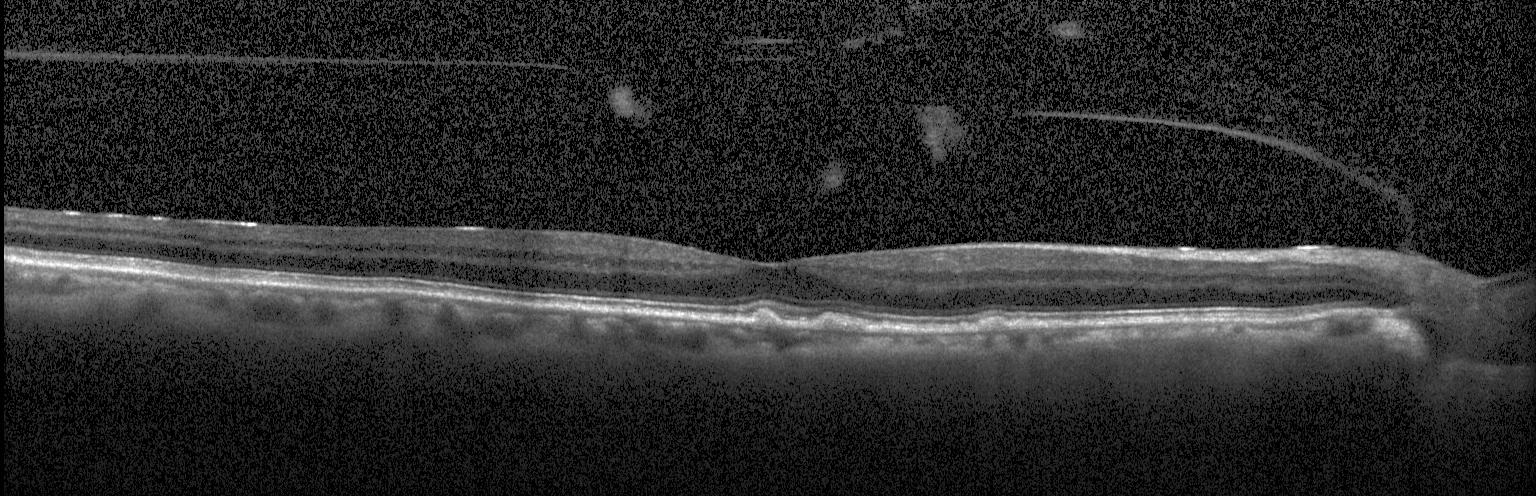 Dx: drusen.